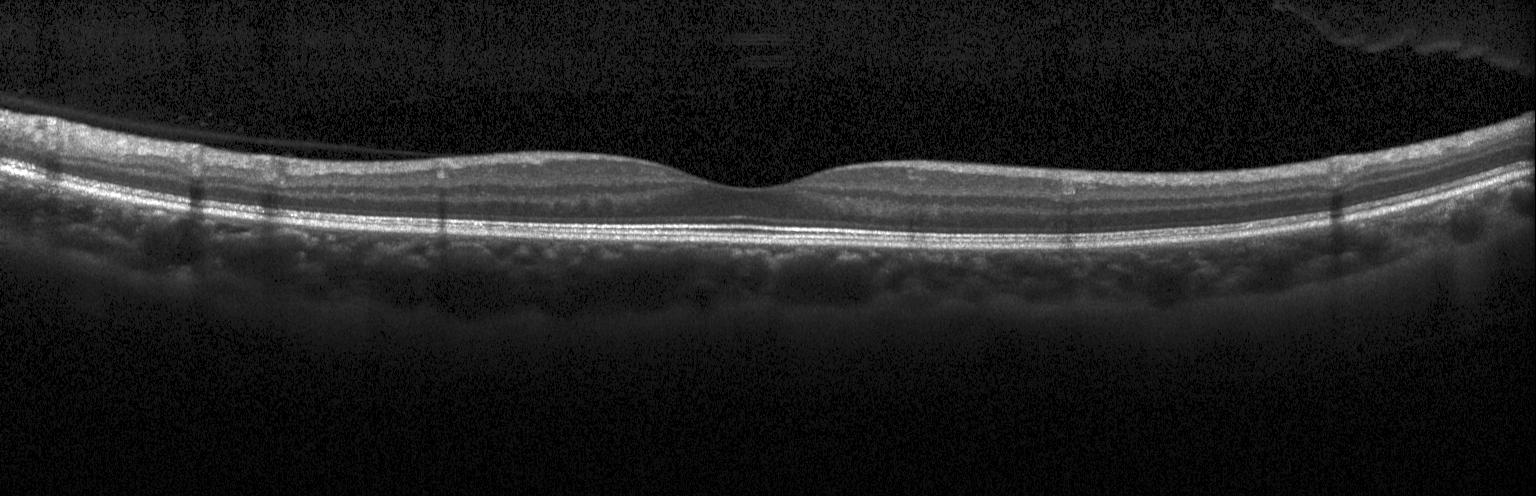

OCT line scan. SD-OCT — Diagnosis: no CNV, no DME, and no drusen.